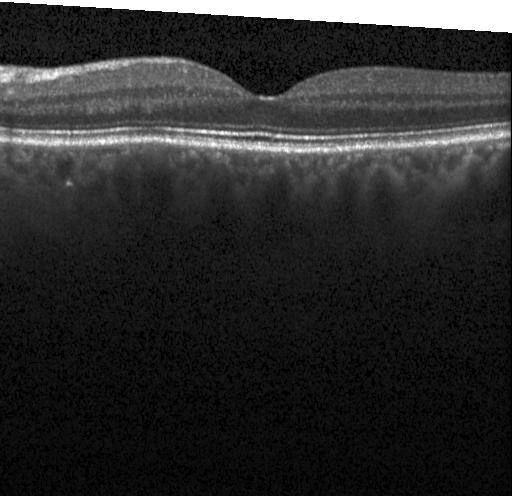 OCT B-scan
Impression: neither CNV, DME, nor drusen.